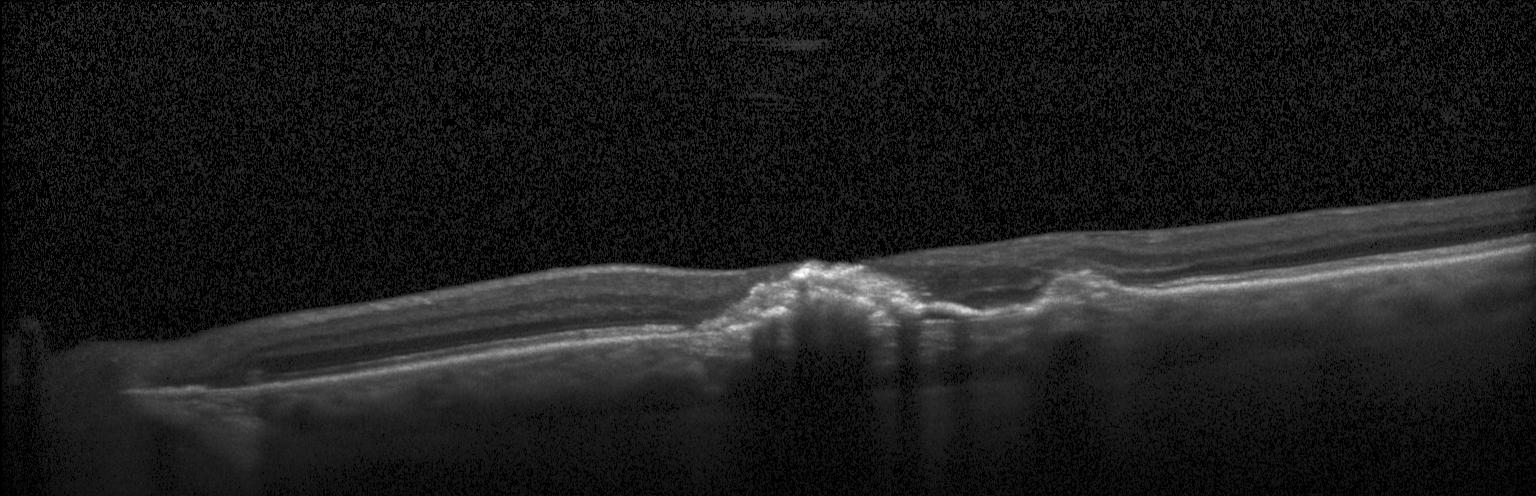

Centered on the fovea, acquired on a Heidelberg Spectralis, OCT B-scan, SD-OCT.
OCT finding: choroidal neovascularization (CNV).